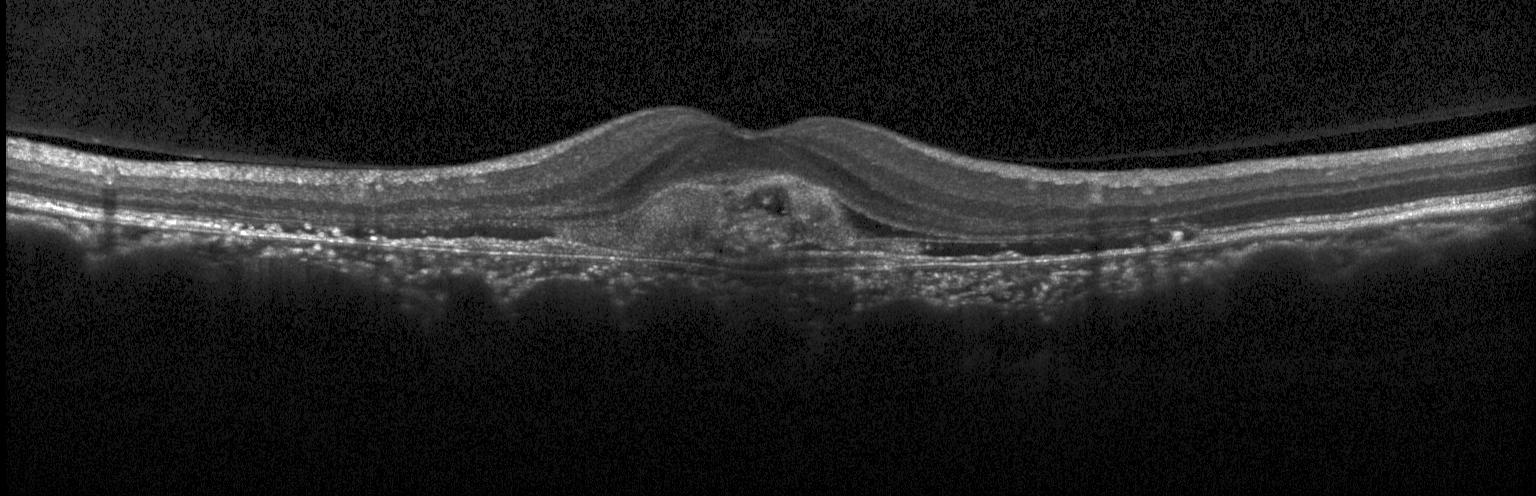

OCT line scan.
The scan shows a choroidal neovascular membrane.